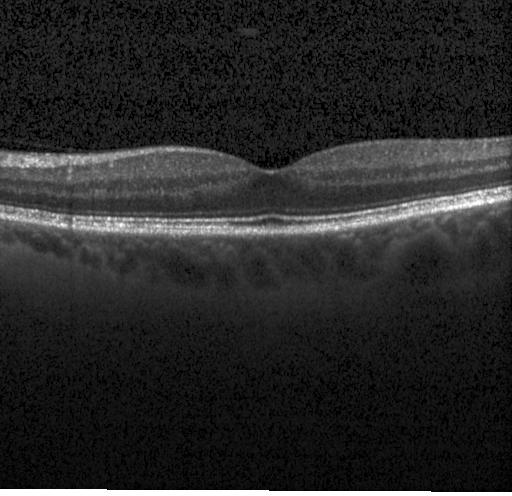
Dx: no choroidal neovascularization, diabetic macular edema, or drusen.